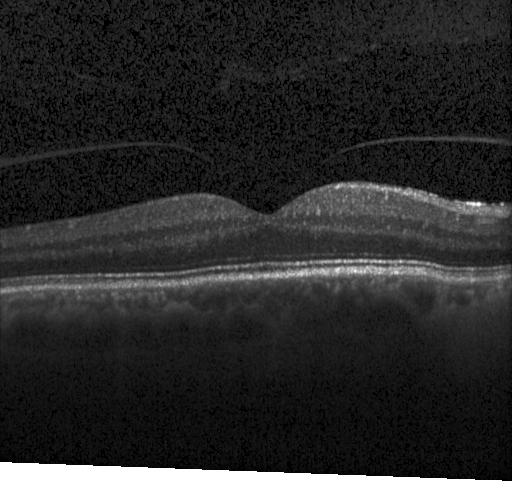
Retinal OCT cross-section showing no evidence of choroidal neovascularization, diabetic macular edema, or drusen.